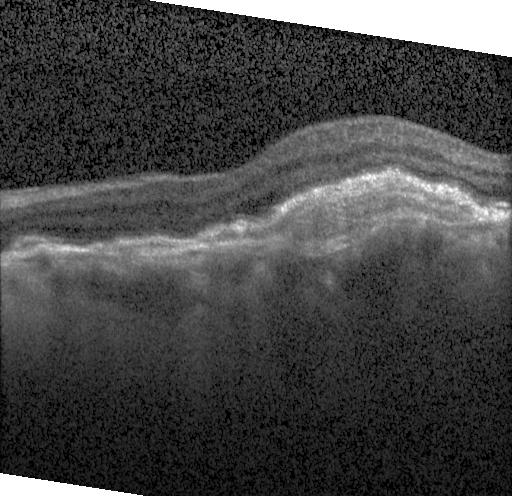

OCT line scan. Assessment: choroidal neovascularization (CNV).